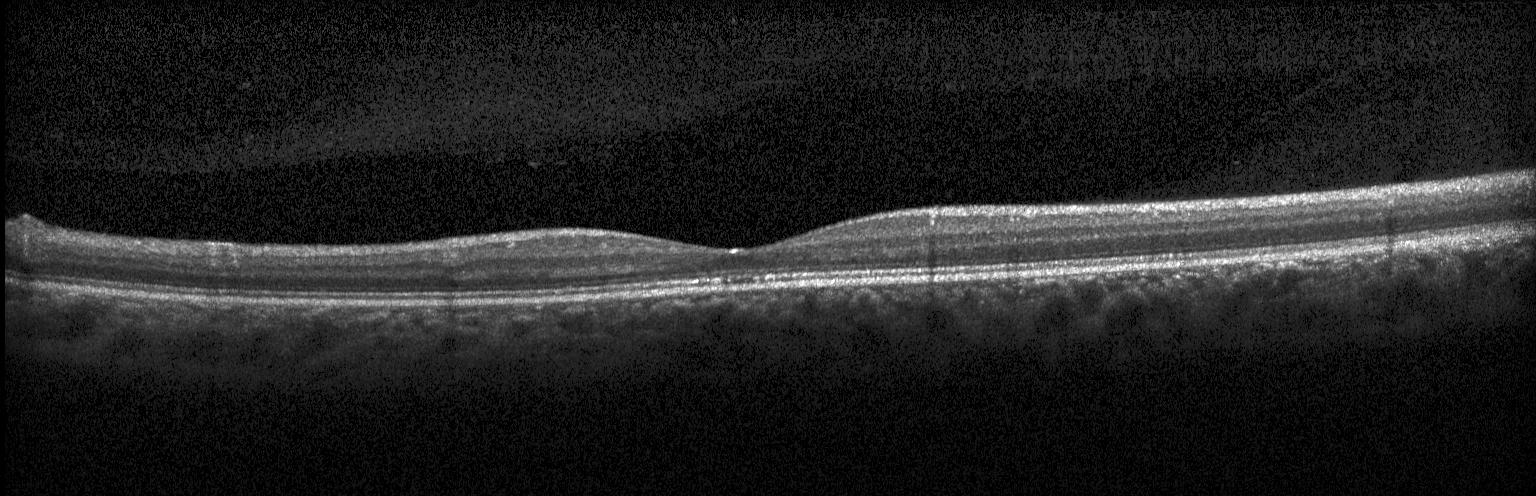
Retinal OCT cross-section; Heidelberg Spectralis OCT system; spectral-domain OCT — The scan shows neither choroidal neovascularization, diabetic macular edema, nor drusen.